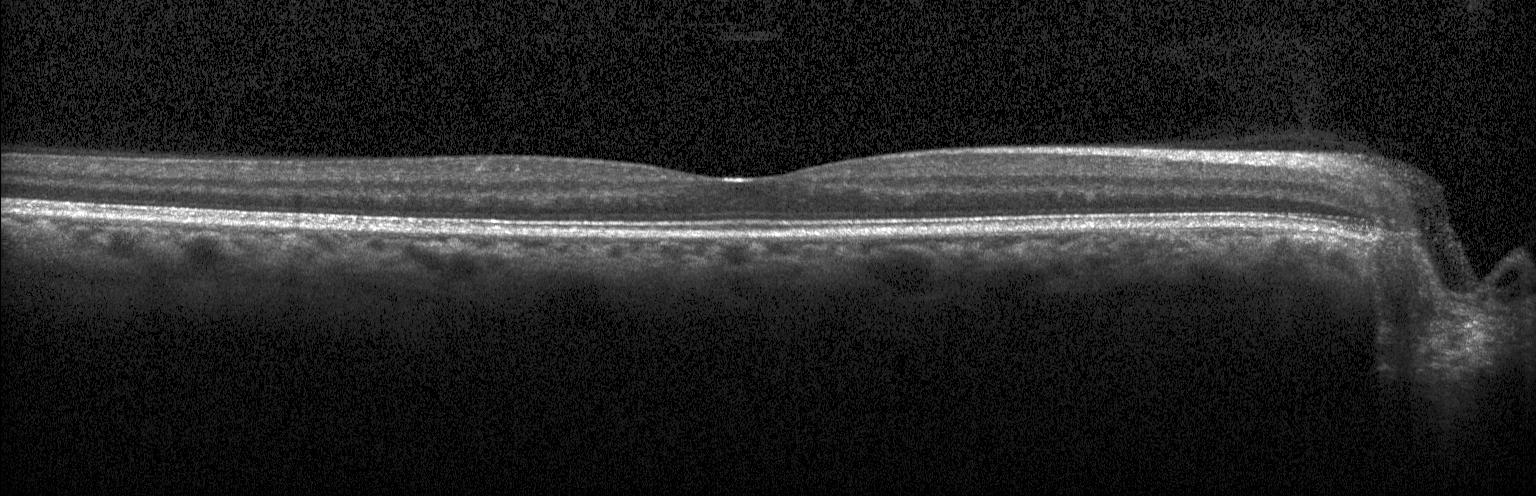
Optical coherence tomography B-scan; instrument: Heidelberg Spectralis; macular scan; SD-OCT — The scan shows no evidence of CNV, DME, or drusen.